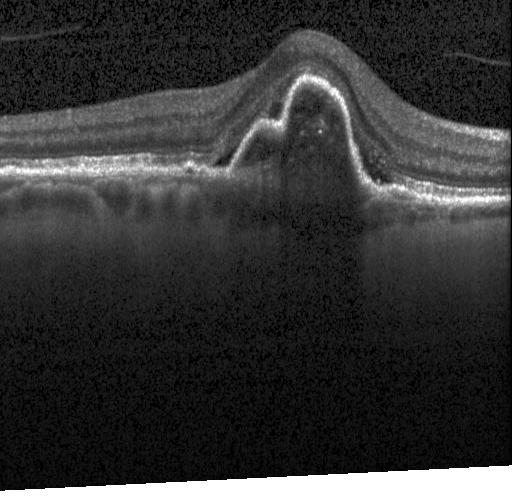

OCT B-scan. Impression: a choroidal neovascular membrane.